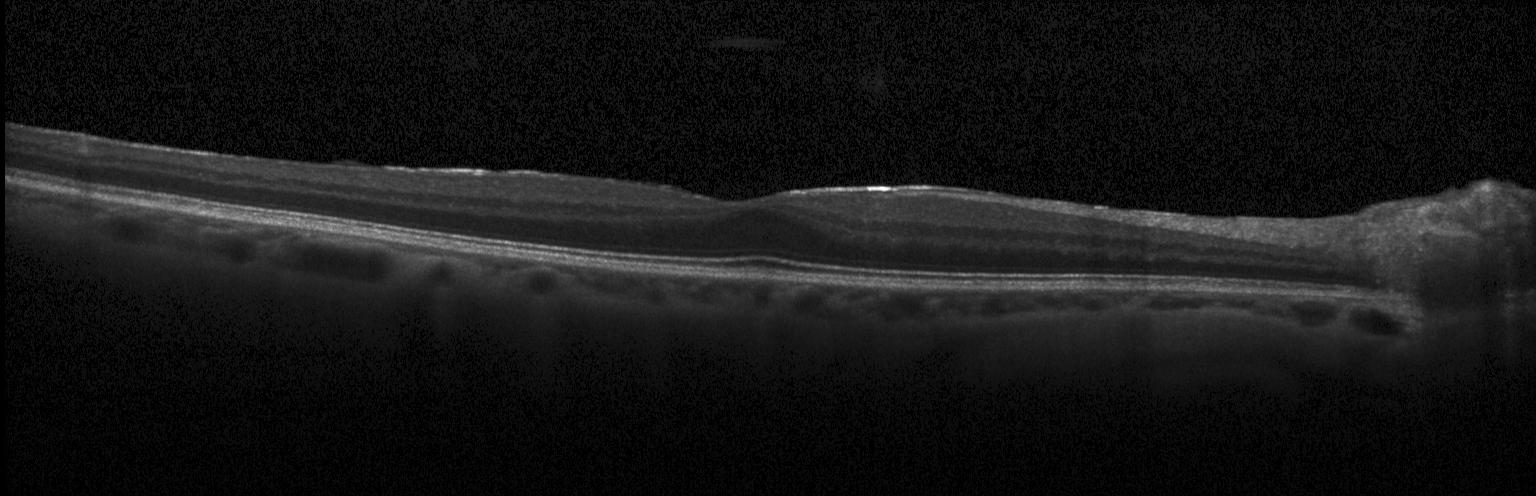

Dx: no choroidal neovascularization, diabetic macular edema, or drusen.